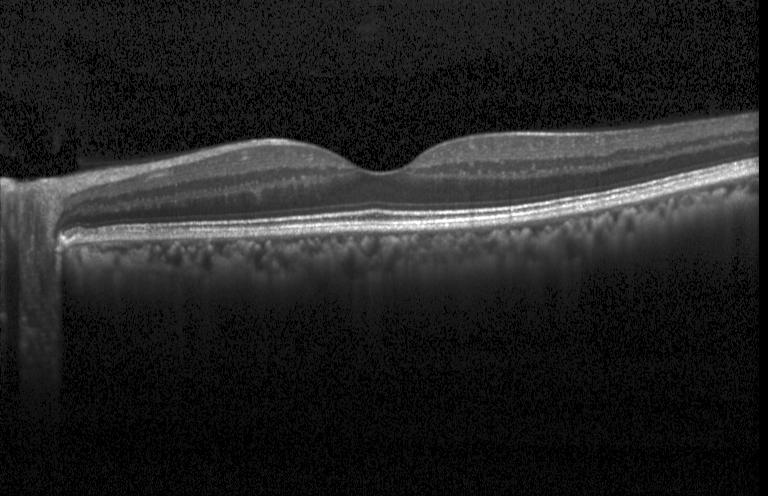 Impression: no evidence of choroidal neovascularization, diabetic macular edema, or drusen.